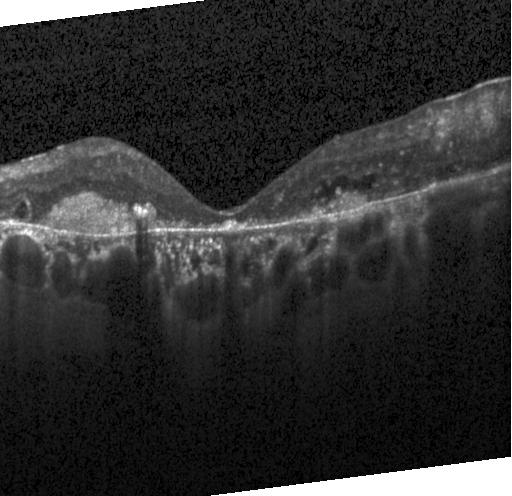

Diagnosis: a choroidal neovascular membrane.